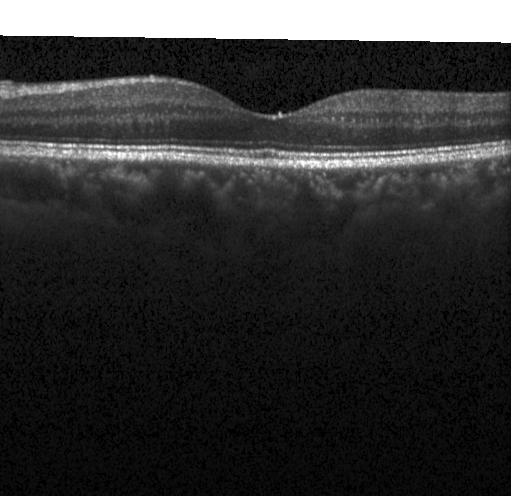
OCT finding: no CNV, no DME, and no drusen.